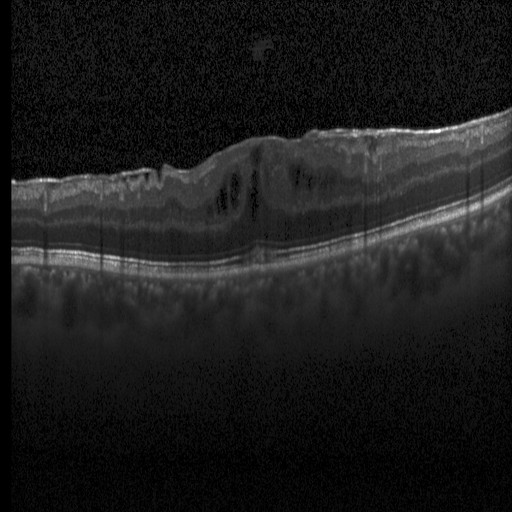
Finding: diabetic macular edema (DME).